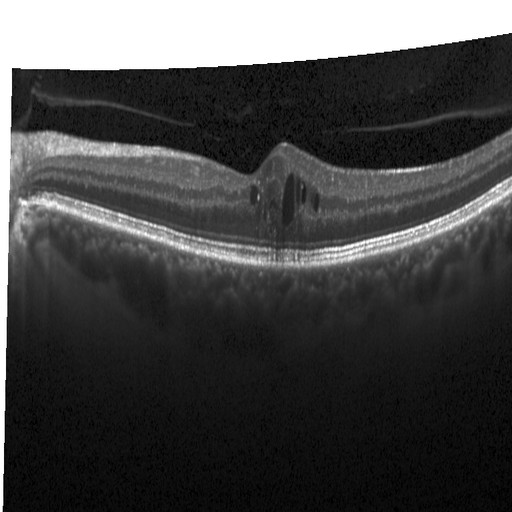 Finding: diabetic macular edema (DME).